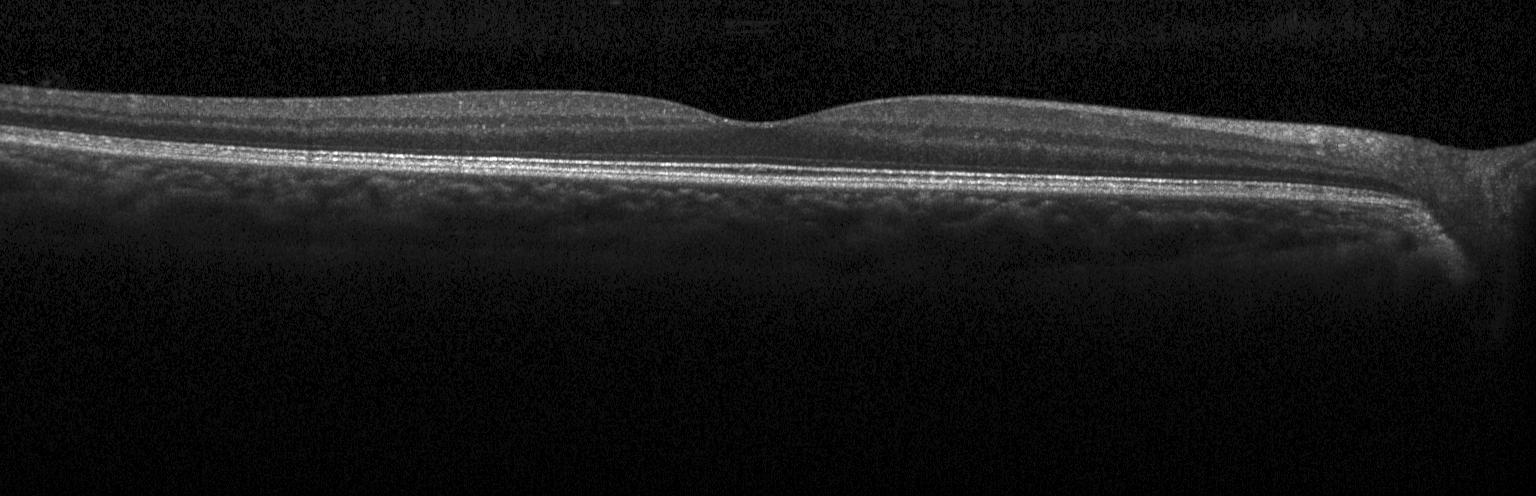 Dx: no choroidal neovascularization, diabetic macular edema, or drusen.